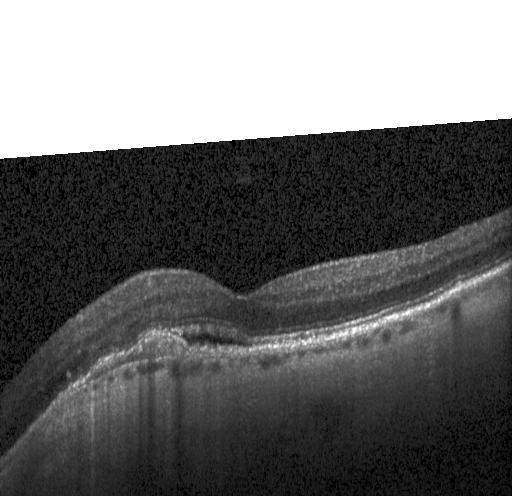

Impression: choroidal neovascularization (CNV).